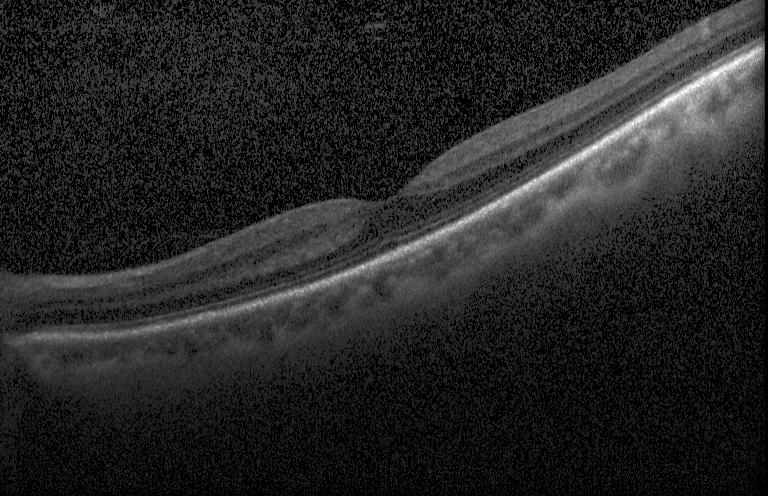

Centered on the fovea, optical coherence tomography B-scan
This B-scan demonstrates no choroidal neovascularization, diabetic macular edema, or drusen.